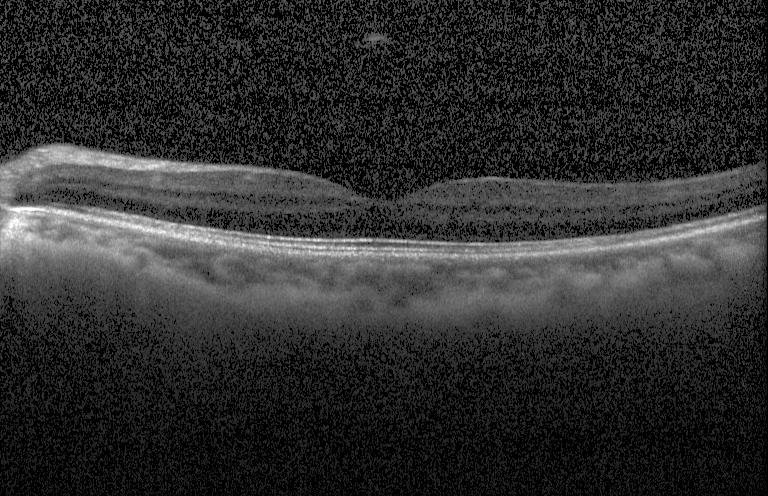

Impression: no choroidal neovascularization, diabetic macular edema, or drusen.